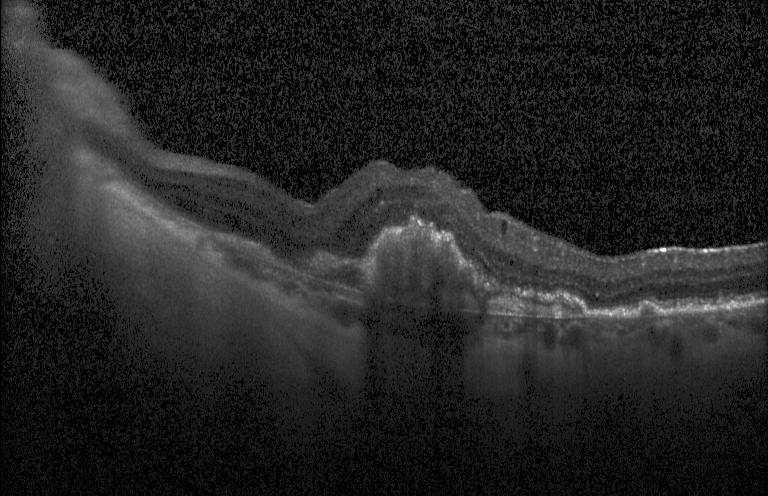

Impression: CNV.